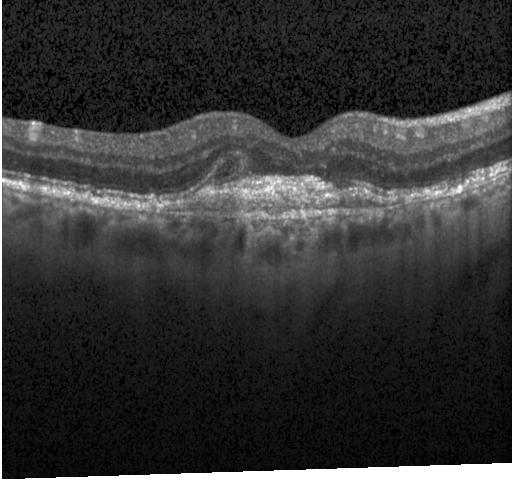

Instrument: Heidelberg Spectralis. Optical coherence tomography B-scan — The scan shows a choroidal neovascular membrane.